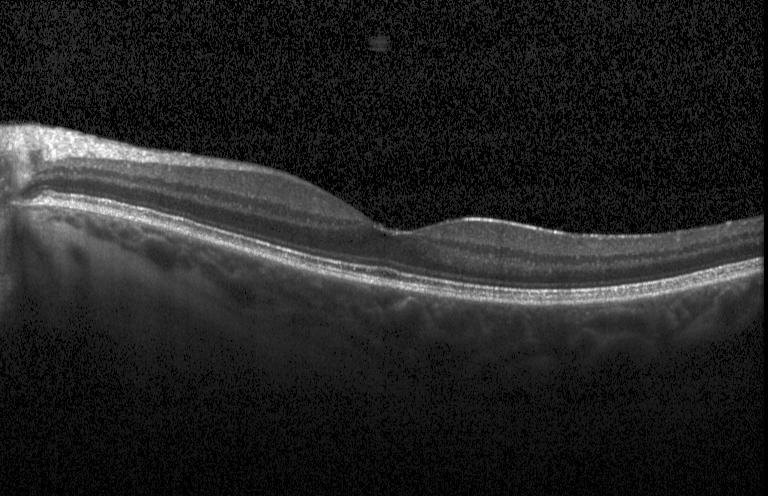 Finding: no choroidal neovascularization, no diabetic macular edema, and no drusen.